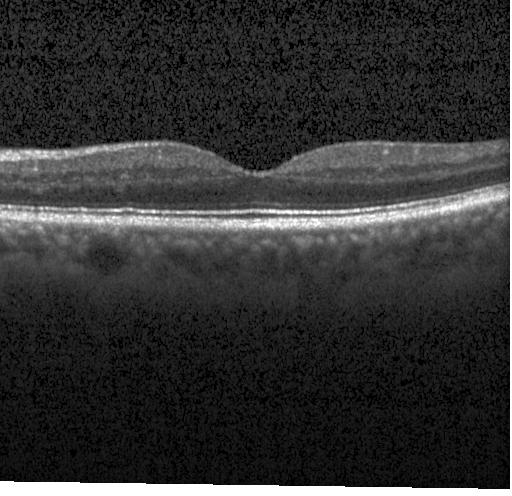

Diagnosis: no choroidal neovascularization, no diabetic macular edema, and no drusen.